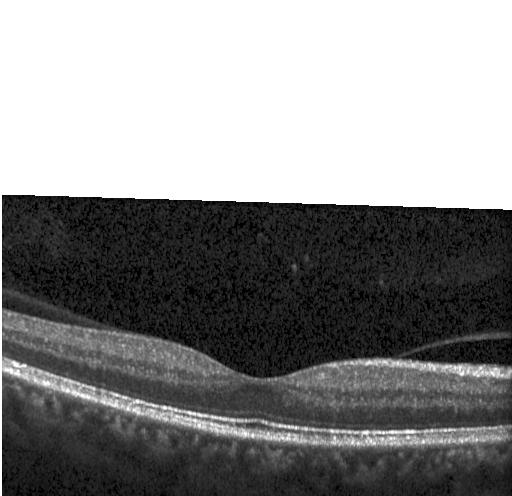 OCT B-scan. Impression: no choroidal neovascularization, diabetic macular edema, or drusen.